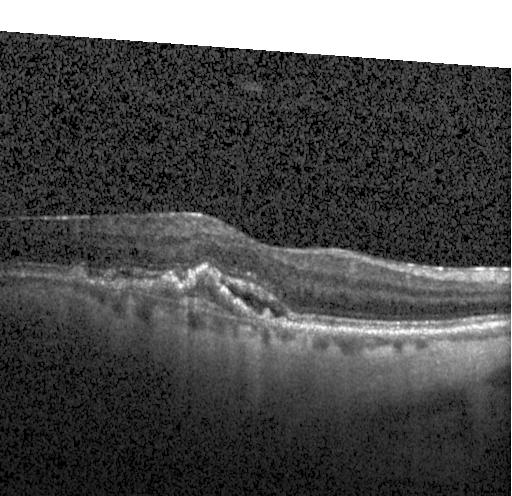

OCT finding: a choroidal neovascular membrane.